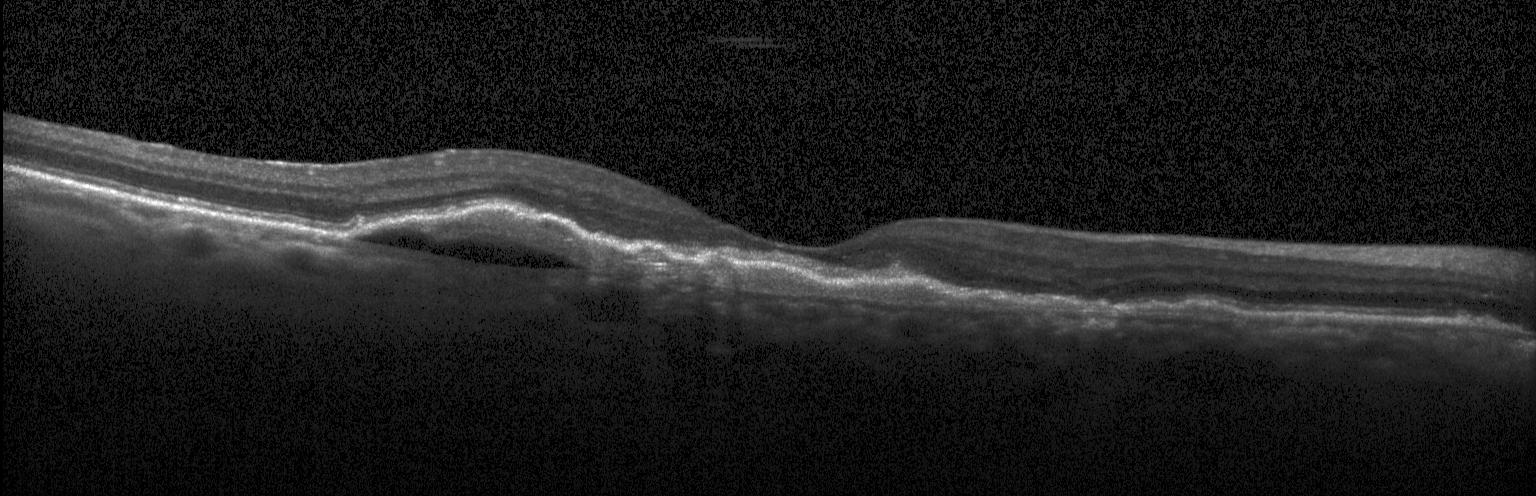
OCT line scan. The scan shows choroidal neovascularization (CNV).